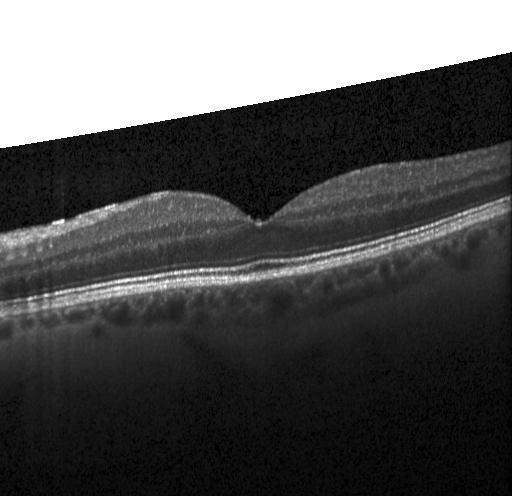
OCT finding: neither choroidal neovascularization, diabetic macular edema, nor drusen.